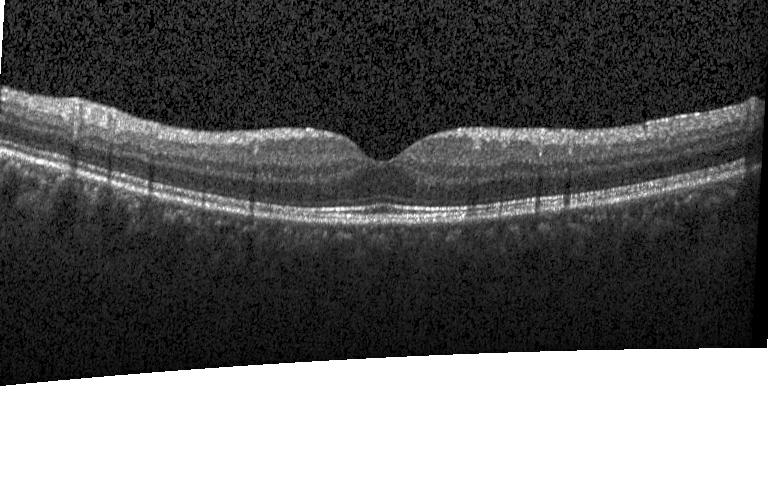

OCT line scan. No choroidal neovascularization, no diabetic macular edema, and no drusen.